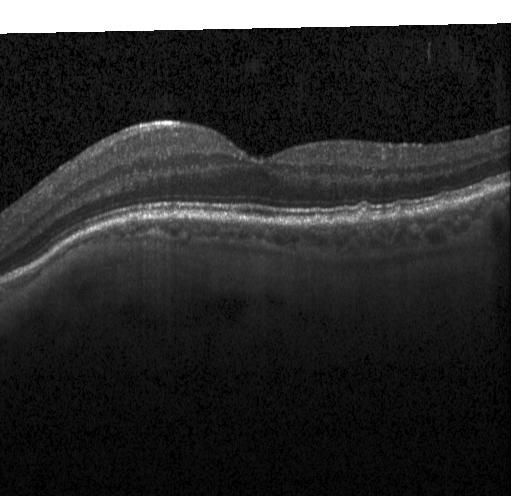
Optical coherence tomography B-scan. Macular OCT: multiple drusen.